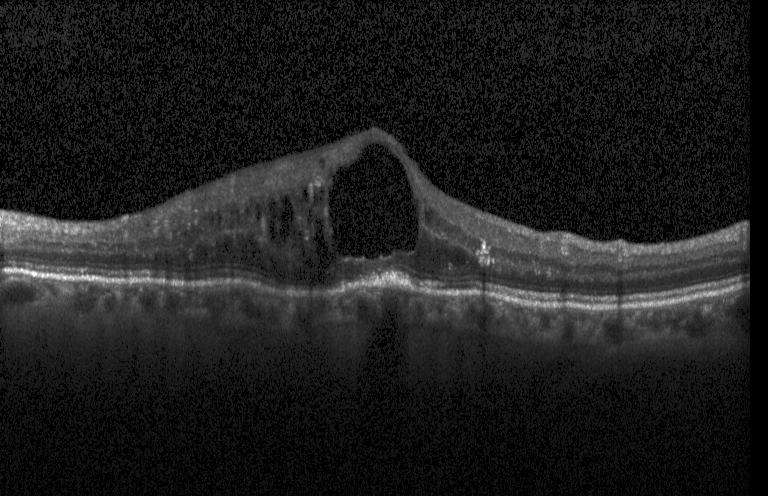

This B-scan demonstrates diabetic macular edema.